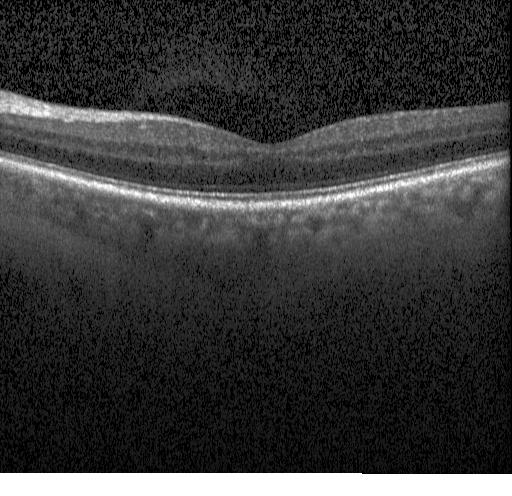

Impression: no choroidal neovascularization, diabetic macular edema, or drusen.